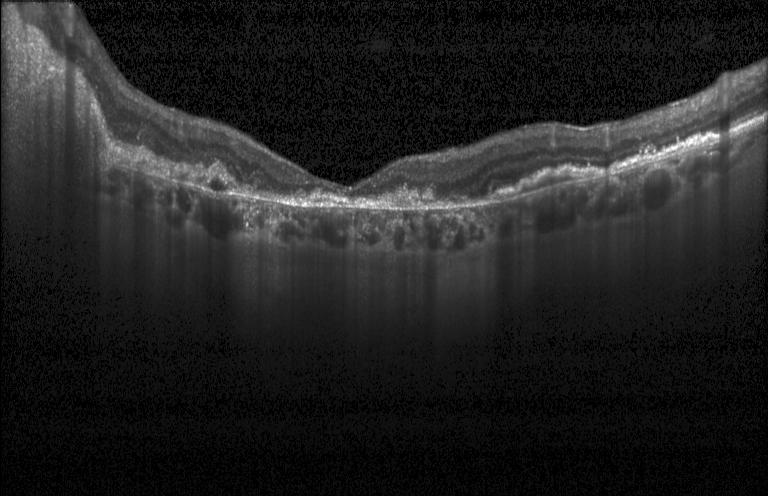
OCT line scan, SD-OCT, acquired on a Heidelberg Spectralis.
Diagnosis: a choroidal neovascular membrane.